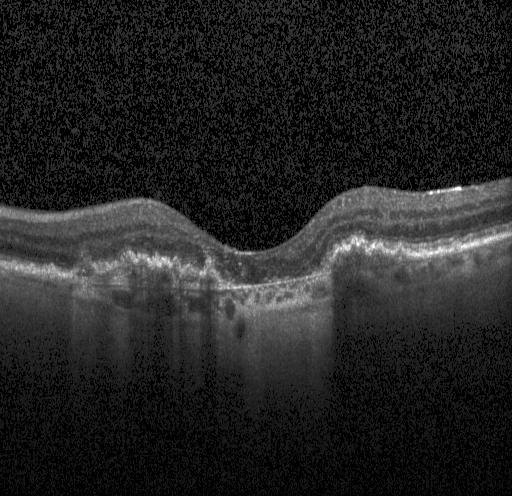

Heidelberg Spectralis; spectral-domain optical coherence tomography; OCT line scan; horizontal scan through the fovea.
Macular OCT: choroidal neovascularization (CNV).